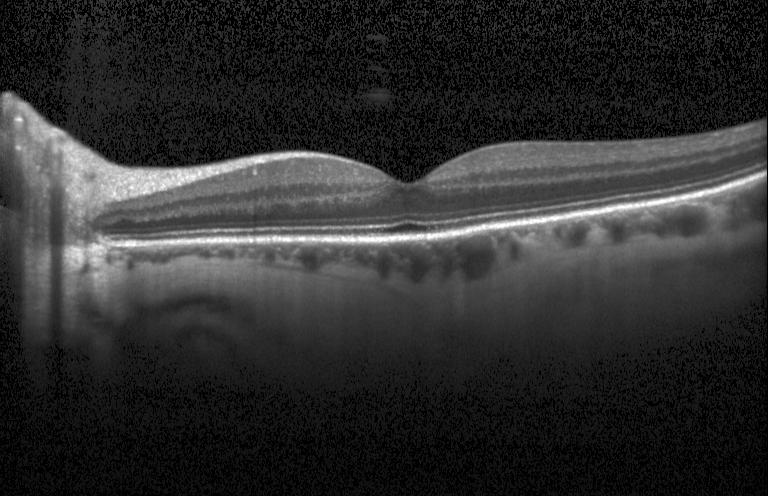

Heidelberg Spectralis · OCT B-scan
Diagnosis: no evidence of CNV, DME, or drusen.